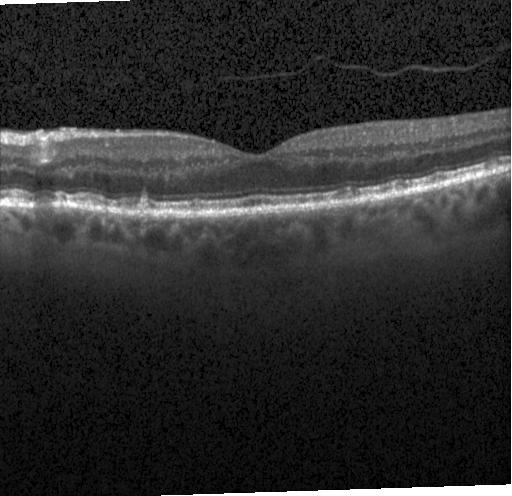

OCT B-scan showing drusen.